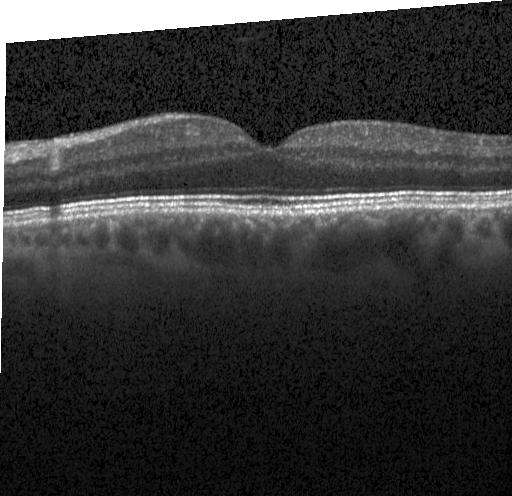 Assessment: no choroidal neovascularization, no diabetic macular edema, and no drusen.